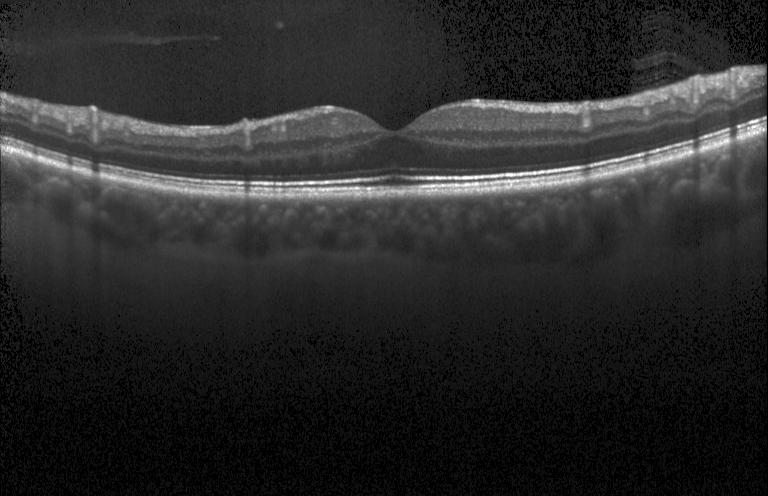
Diagnosis: no choroidal neovascularization, no diabetic macular edema, and no drusen.